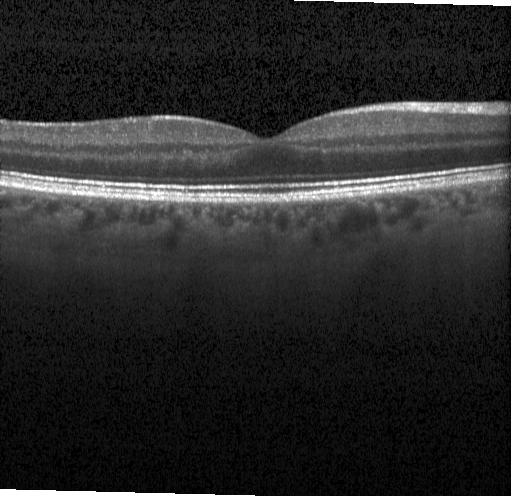

Centered on the fovea, Heidelberg Spectralis OCT system, spectral-domain optical coherence tomography, OCT line scan — Diagnosis: no CNV, DME, or drusen.